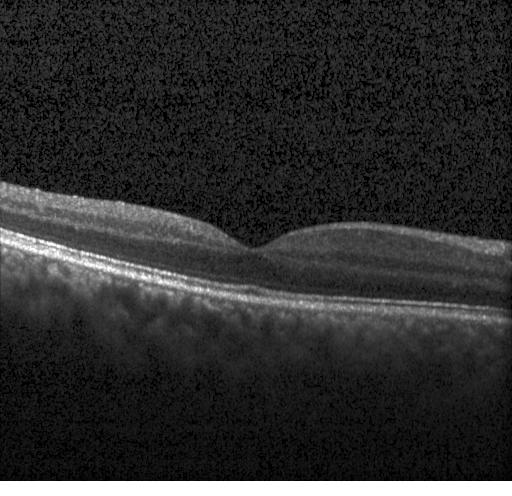 This B-scan demonstrates no evidence of CNV, DME, or drusen.